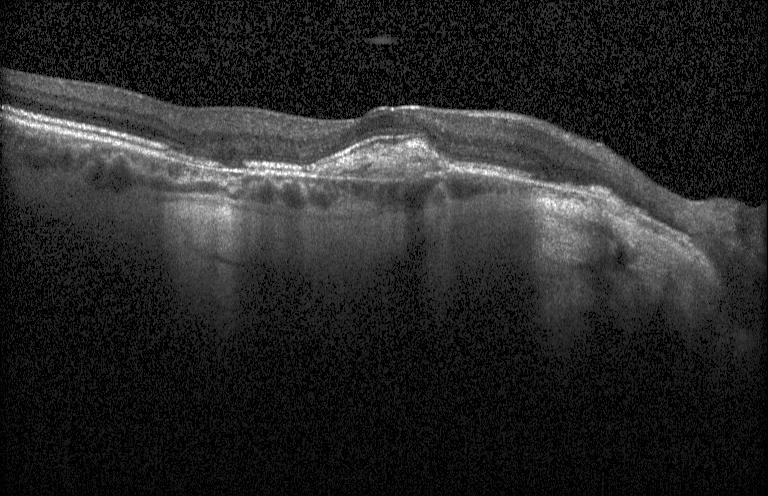
Optical coherence tomography scan; spectral-domain optical coherence tomography
The scan shows a choroidal neovascular membrane.